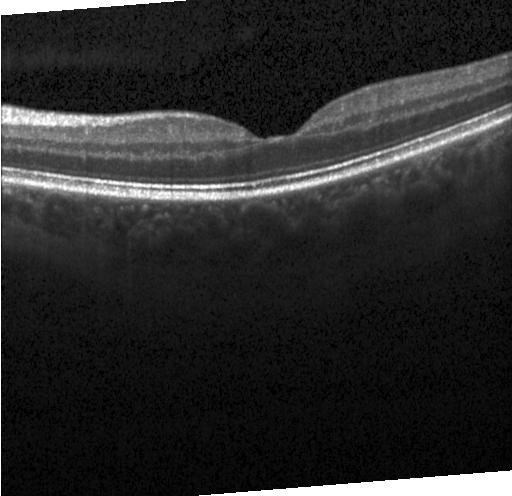

Finding: no evidence of choroidal neovascularization, diabetic macular edema, or drusen.